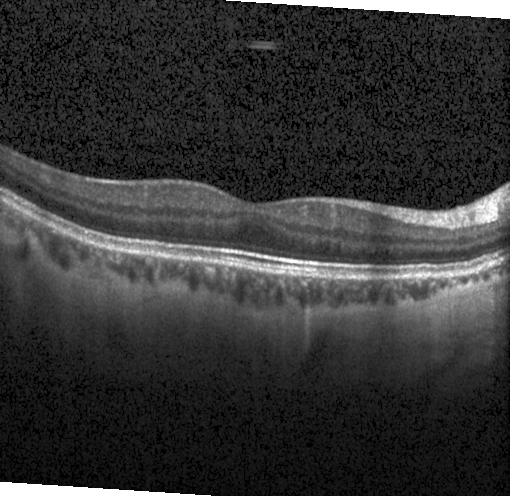
Impression: no choroidal neovascularization, no diabetic macular edema, and no drusen.